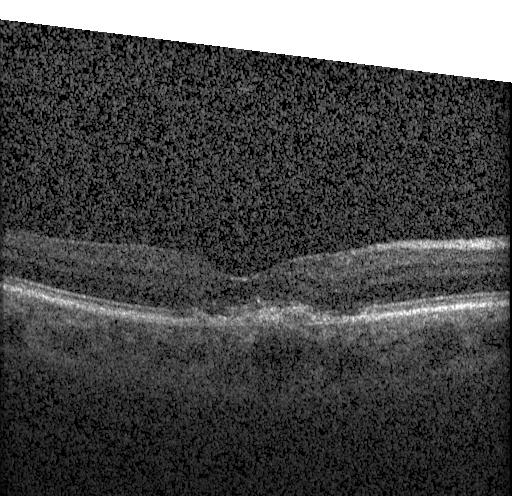

OCT line scan; through the macula; SD-OCT.
Dx: CNV.